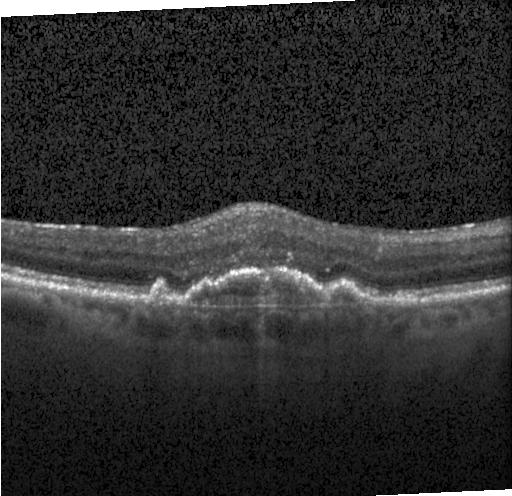
Retinal OCT cross-section showing choroidal neovascularization.